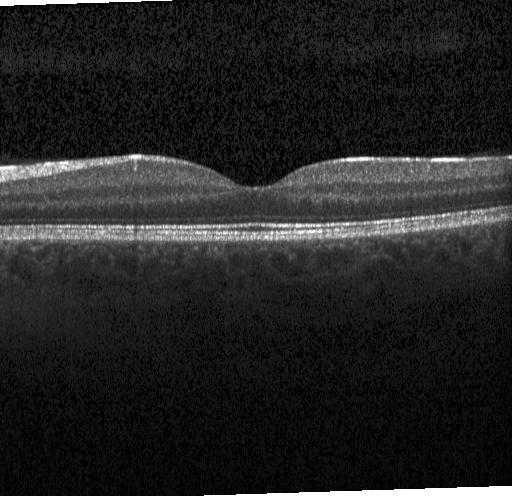 OCT B-scan. SD-OCT. Heidelberg Spectralis
The scan shows no CNV, DME, or drusen.